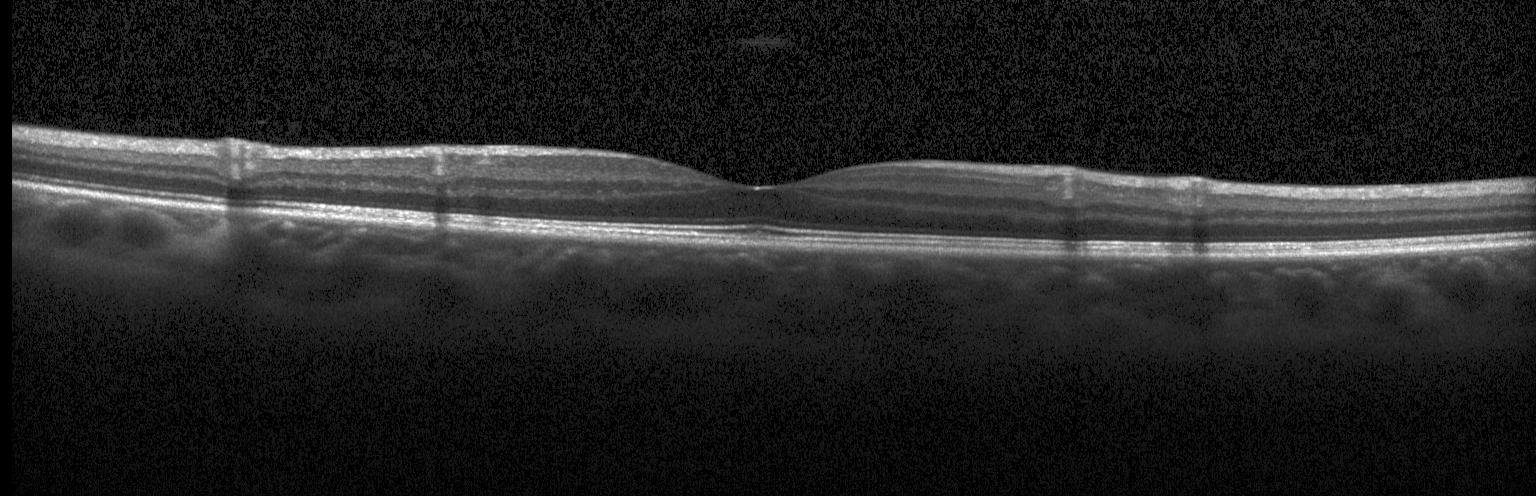 OCT line scan; through the macula — No CNV, no DME, and no drusen.